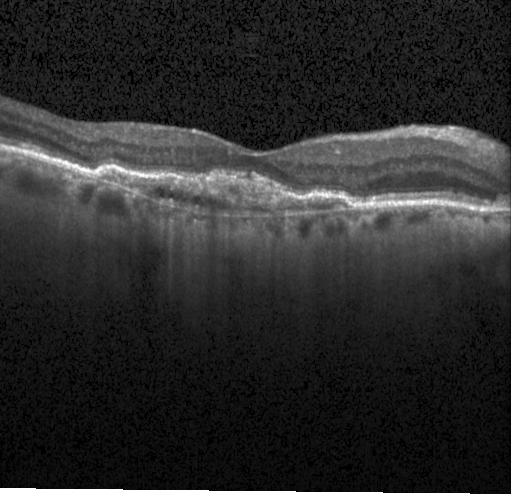
SD-OCT · retinal OCT cross-section · macular scan
Impression: choroidal neovascularization (CNV).